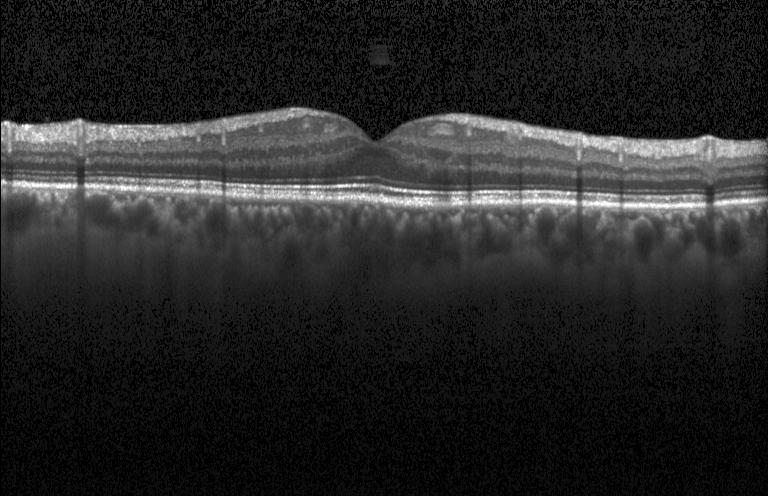
Optical coherence tomography B-scan · horizontal scan through the fovea · acquired on a Heidelberg Spectralis
Finding: no evidence of choroidal neovascularization, diabetic macular edema, or drusen.